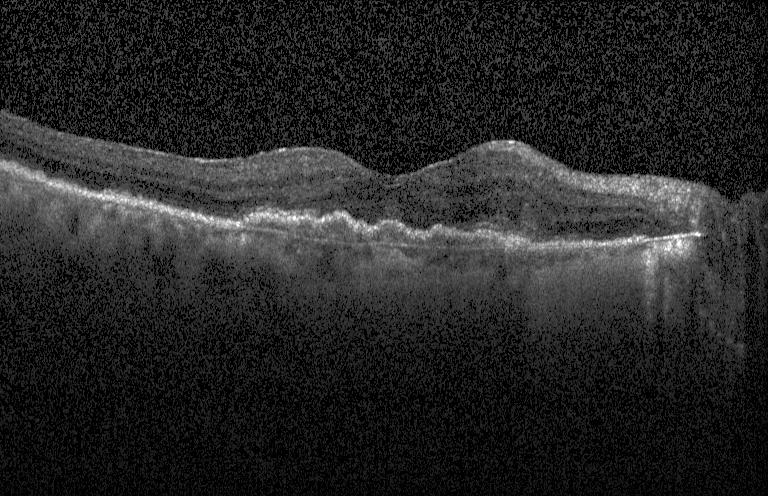 Spectral-domain OCT B-scan: choroidal neovascularization (CNV).